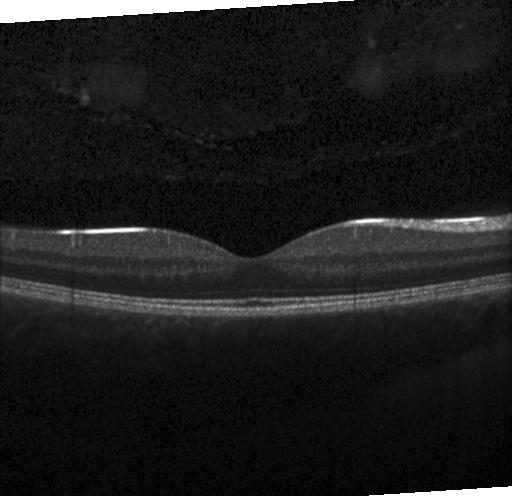
Heidelberg Spectralis · retinal OCT cross-section · spectral-domain optical coherence tomography · through the macula.
Dx: no evidence of choroidal neovascularization, diabetic macular edema, or drusen.